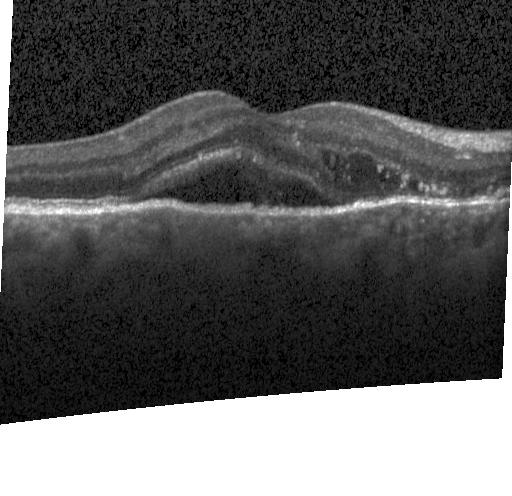 Optical coherence tomography scan. SD-OCT
Finding: CNV.